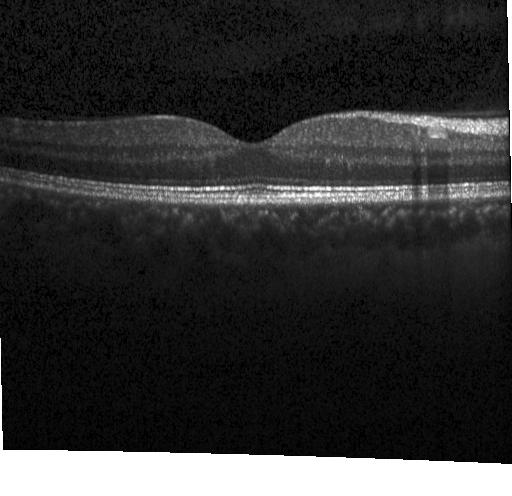

Retinal OCT cross-section. Macular scan
Dx: neither choroidal neovascularization, diabetic macular edema, nor drusen.